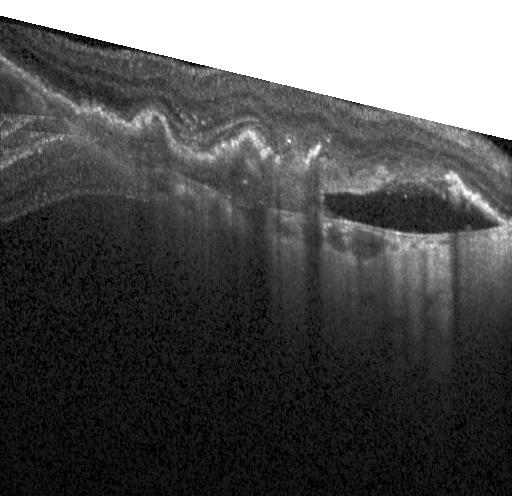 Instrument: Heidelberg Spectralis; spectral-domain optical coherence tomography; optical coherence tomography scan; centered on the fovea
Assessment: a choroidal neovascular membrane.